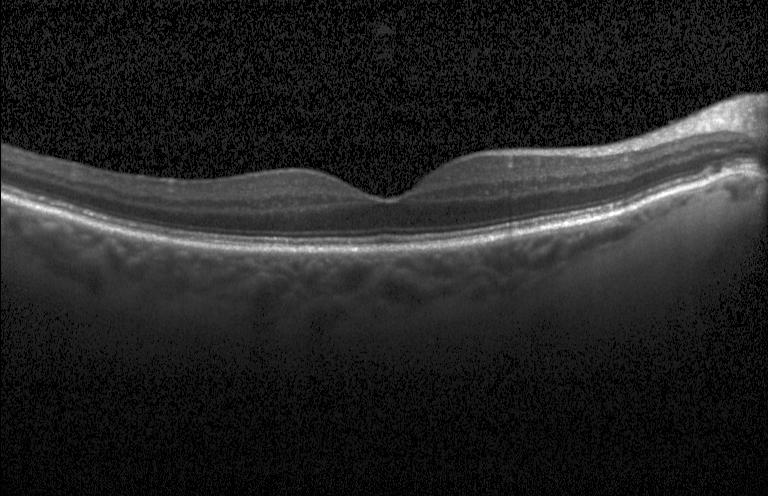 OCT finding: no choroidal neovascularization, diabetic macular edema, or drusen.